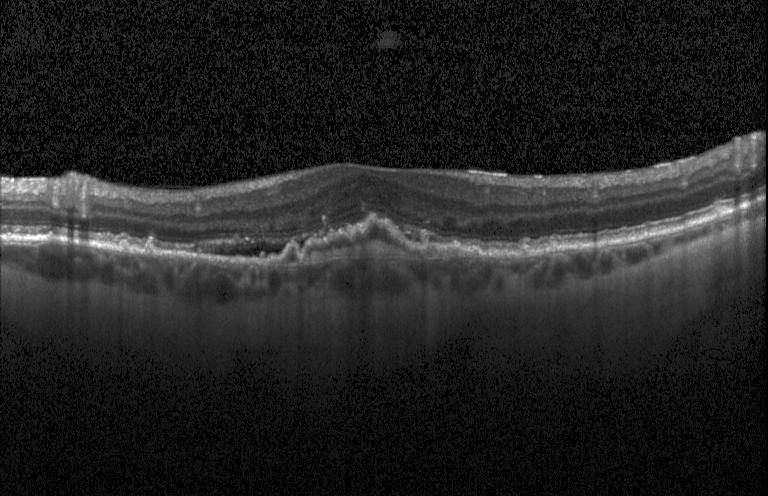 Spectral-domain OCT B-scan: choroidal neovascularization (CNV).